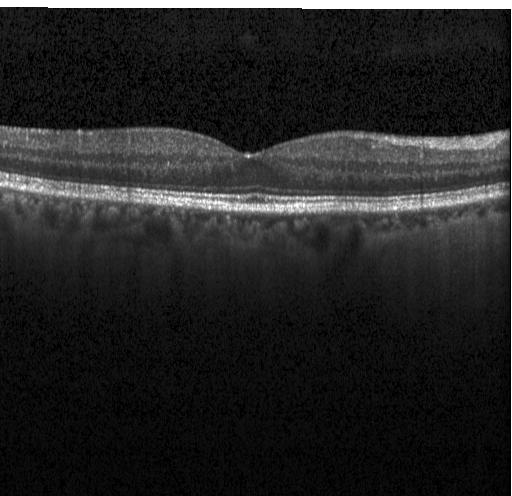
OCT line scan.
Macular OCT: neither choroidal neovascularization, diabetic macular edema, nor drusen.